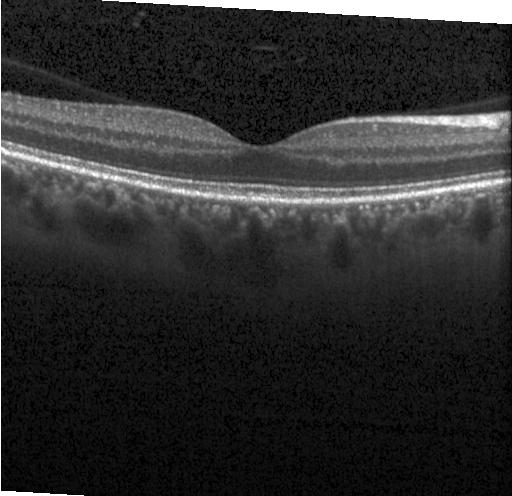 Optical coherence tomography scan; spectral-domain OCT; Heidelberg Spectralis
Impression: no choroidal neovascularization, no diabetic macular edema, and no drusen.